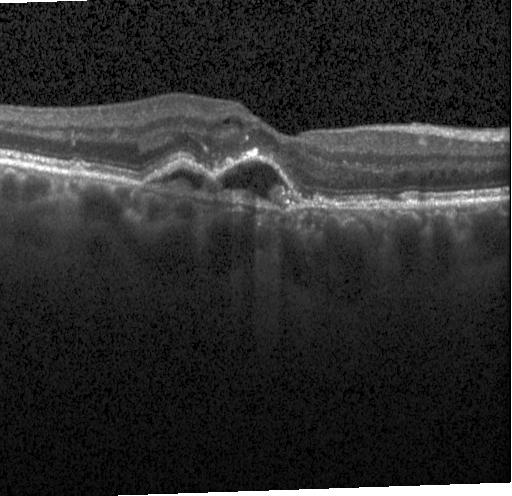

Spectral-domain OCT. OCT B-scan. Fovea-centered. Finding: a choroidal neovascular membrane.